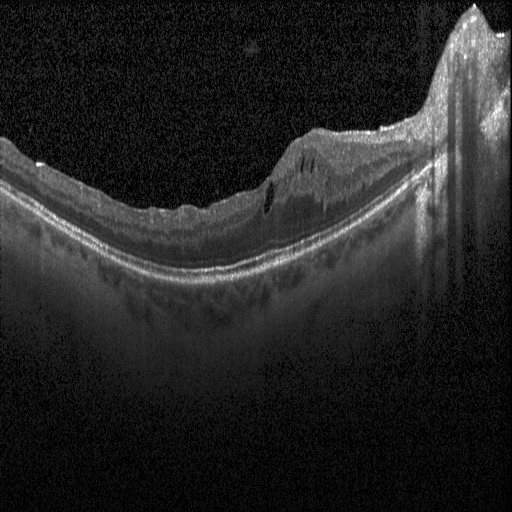
OCT scan showing DME.